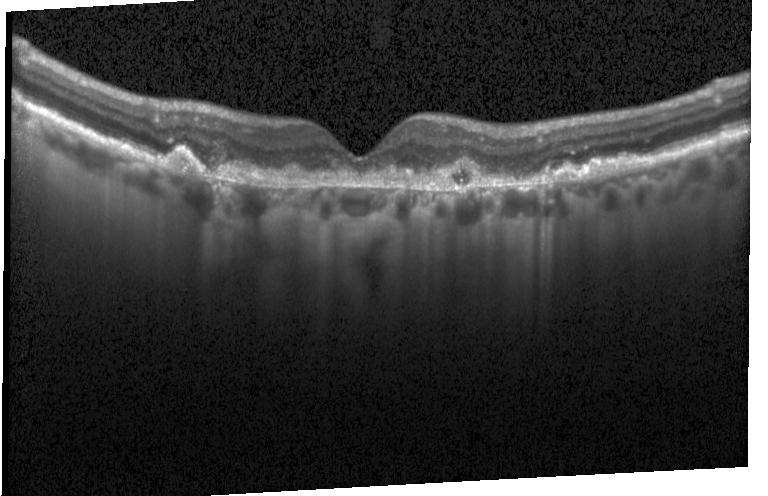

Finding: a choroidal neovascular membrane.